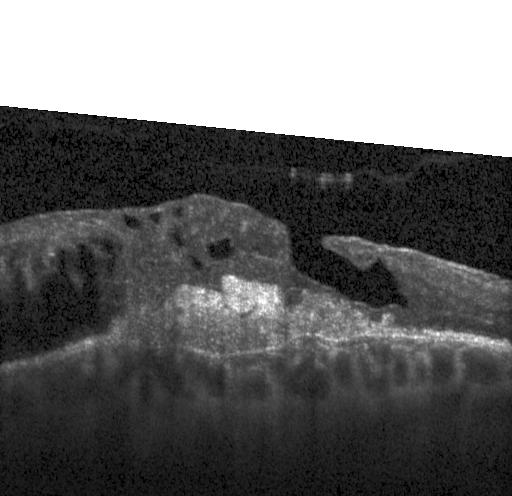

Centered on the fovea. SD-OCT. Heidelberg Spectralis OCT system. Retinal OCT B-scan.
OCT finding: CNV.